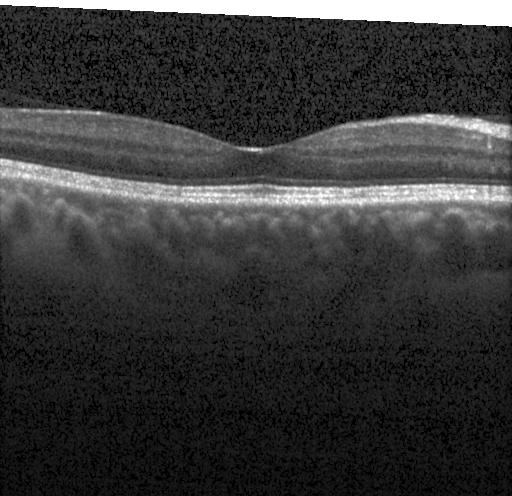
Centered on the fovea; spectral-domain OCT; Heidelberg Spectralis OCT system; optical coherence tomography scan.
Diagnosis: no CNV, DME, or drusen.